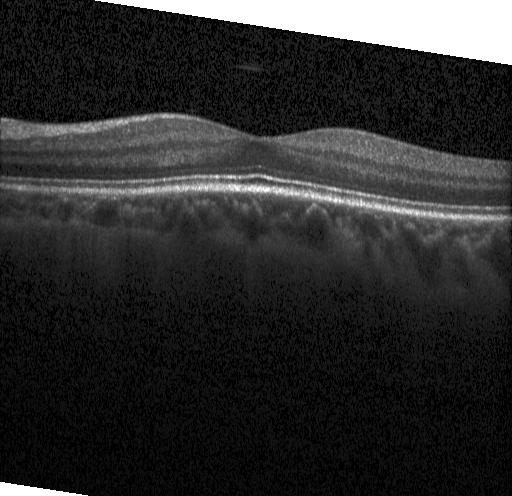
Optical coherence tomography B-scan · instrument: Heidelberg Spectralis · spectral-domain optical coherence tomography.
Impression: neither CNV, DME, nor drusen.